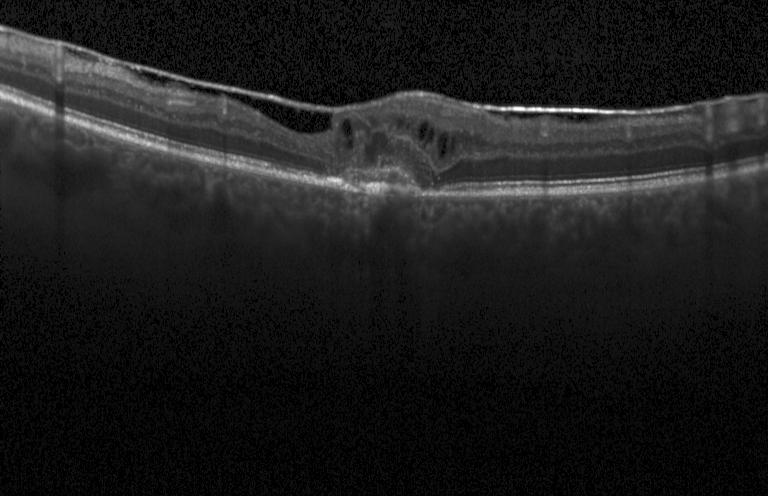

OCT finding: CNV.